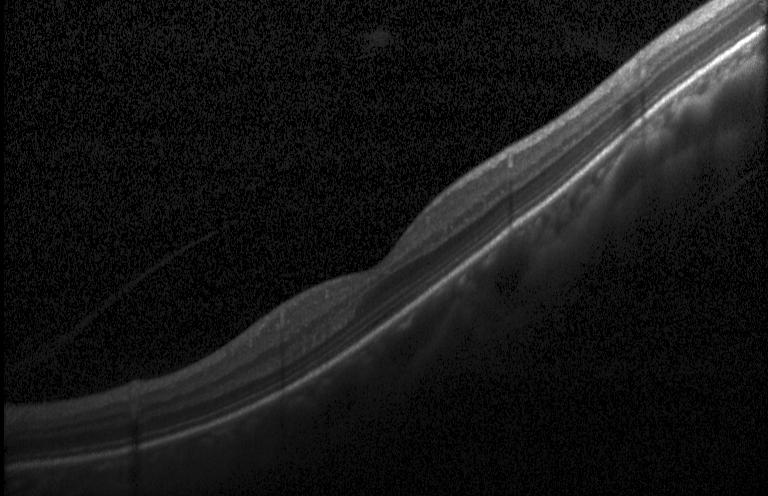
Macular scan · acquired on a Heidelberg Spectralis · optical coherence tomography scan.
This B-scan demonstrates no choroidal neovascularization, no diabetic macular edema, and no drusen.